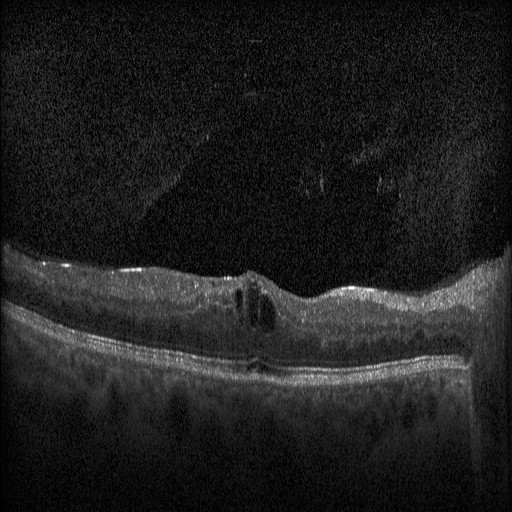

This B-scan demonstrates diabetic macular edema (DME).